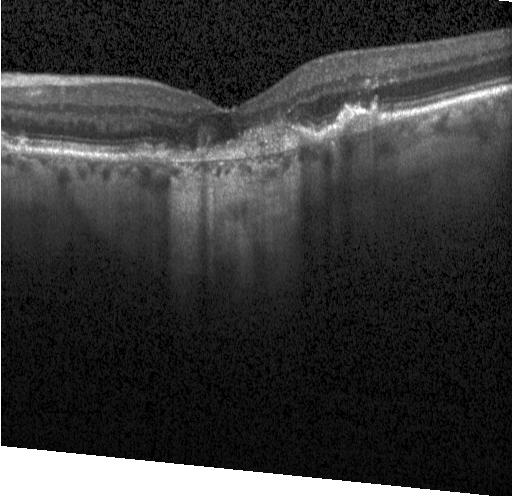
Heidelberg Spectralis OCT system, optical coherence tomography B-scan.
The scan shows a choroidal neovascular membrane.